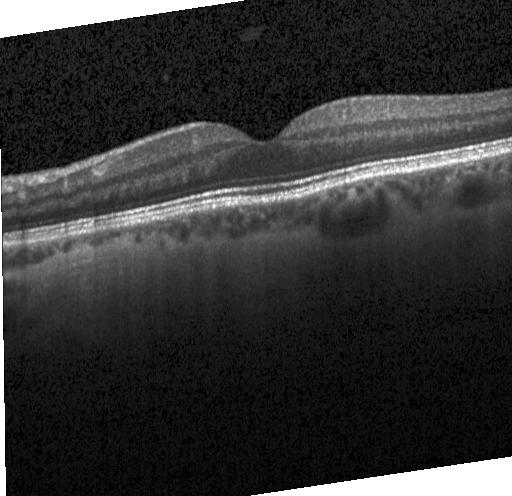
Instrument: Heidelberg Spectralis. Retinal OCT B-scan. Through the macula
This B-scan demonstrates neither choroidal neovascularization, diabetic macular edema, nor drusen.